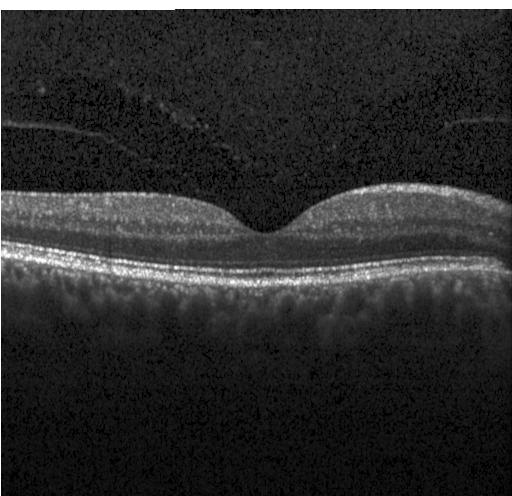
Optical coherence tomography scan. Through the macula. Heidelberg Spectralis OCT system — Diagnosis: no evidence of choroidal neovascularization, diabetic macular edema, or drusen.